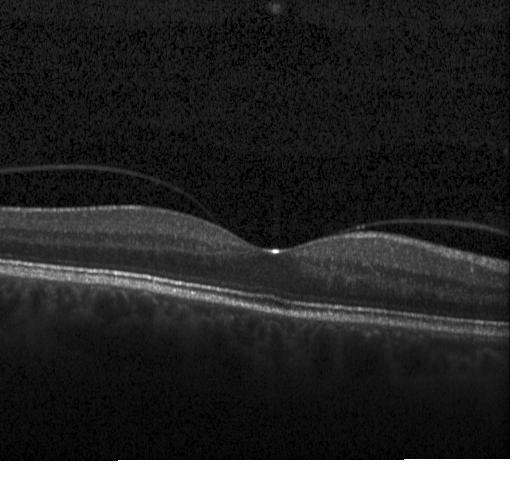 Diagnosis: no choroidal neovascularization, diabetic macular edema, or drusen.